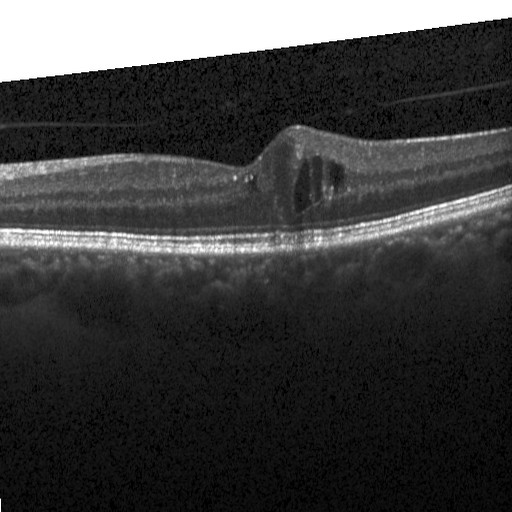 Diagnosis: diabetic macular edema (DME).